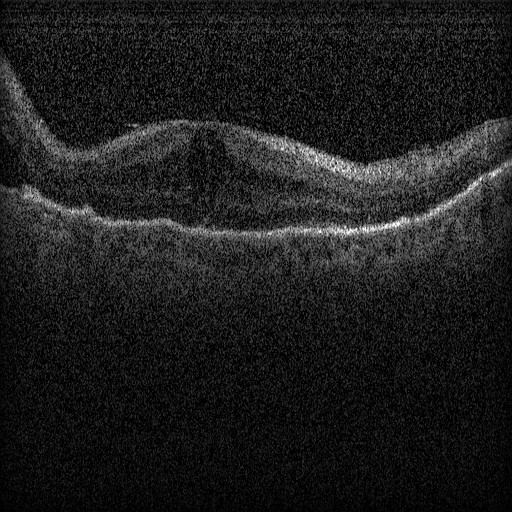

Retinal OCT B-scan. Diagnosis: DME.